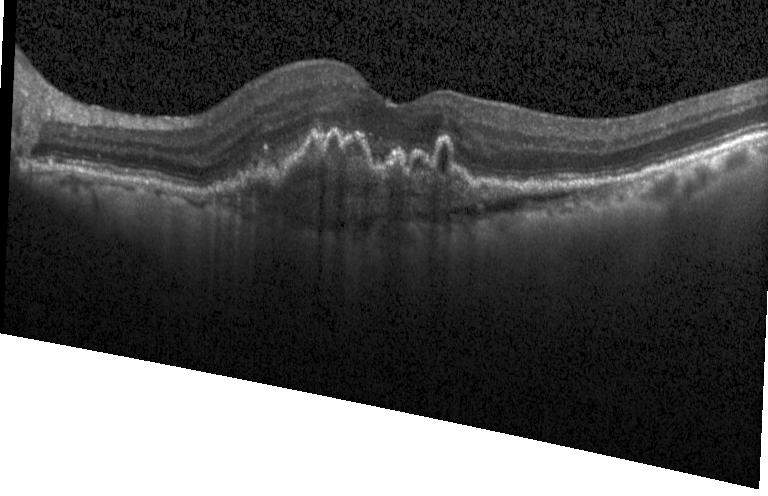 Impression: CNV.